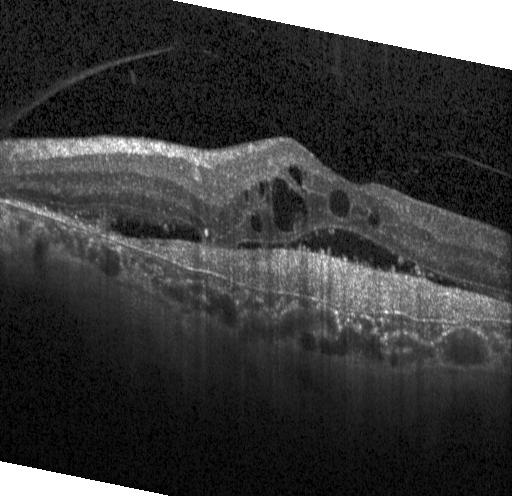 OCT B-scan
Finding: choroidal neovascularization (CNV).